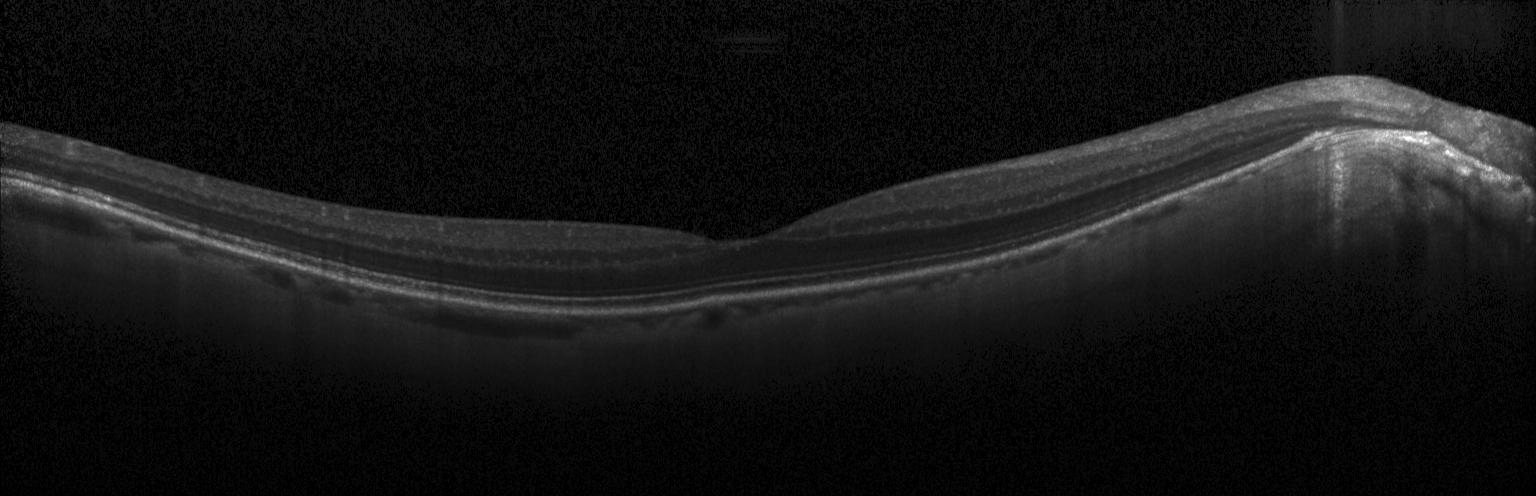

OCT B-scan. Spectral-domain optical coherence tomography. OCT finding: no CNV, no DME, and no drusen.